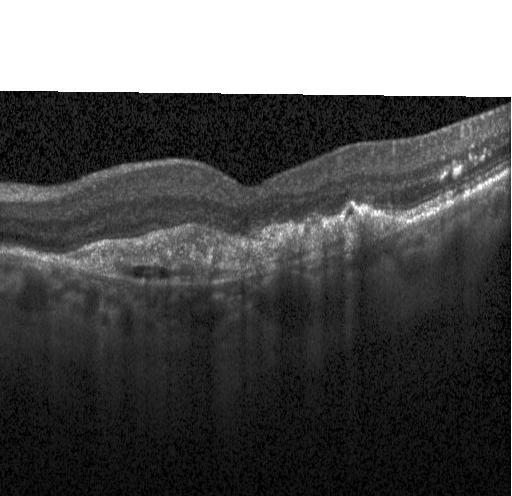 OCT line scan — A choroidal neovascular membrane.